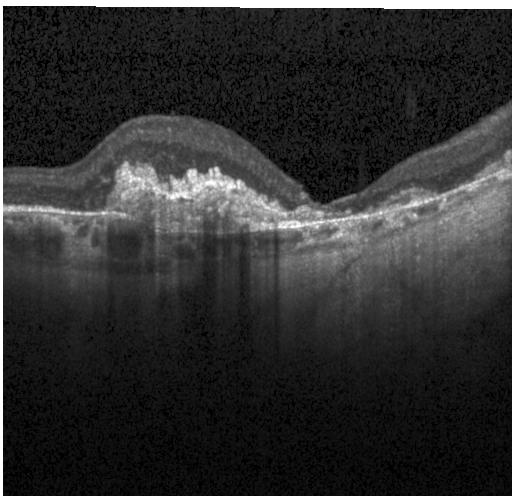
Optical coherence tomography scan. Acquired on a Heidelberg Spectralis. SD-OCT
Finding: CNV.